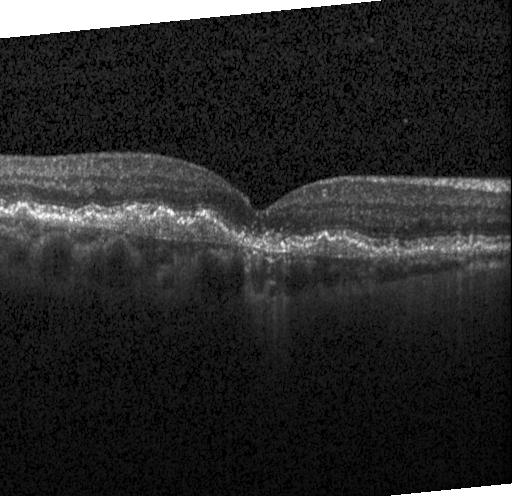
Spectral-domain OCT; optical coherence tomography B-scan; Heidelberg Spectralis OCT system
Impression: a choroidal neovascular membrane.